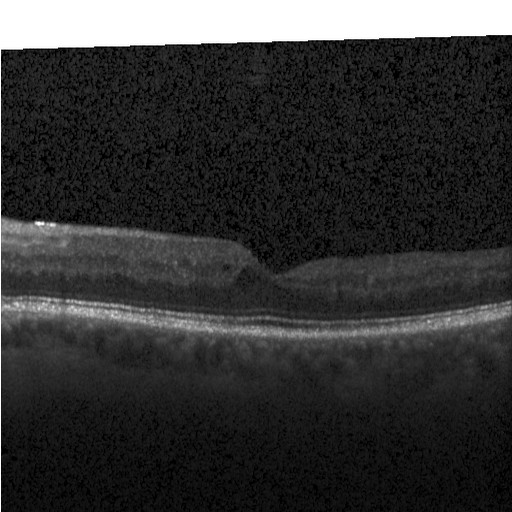

Diagnosis: diabetic macular edema.